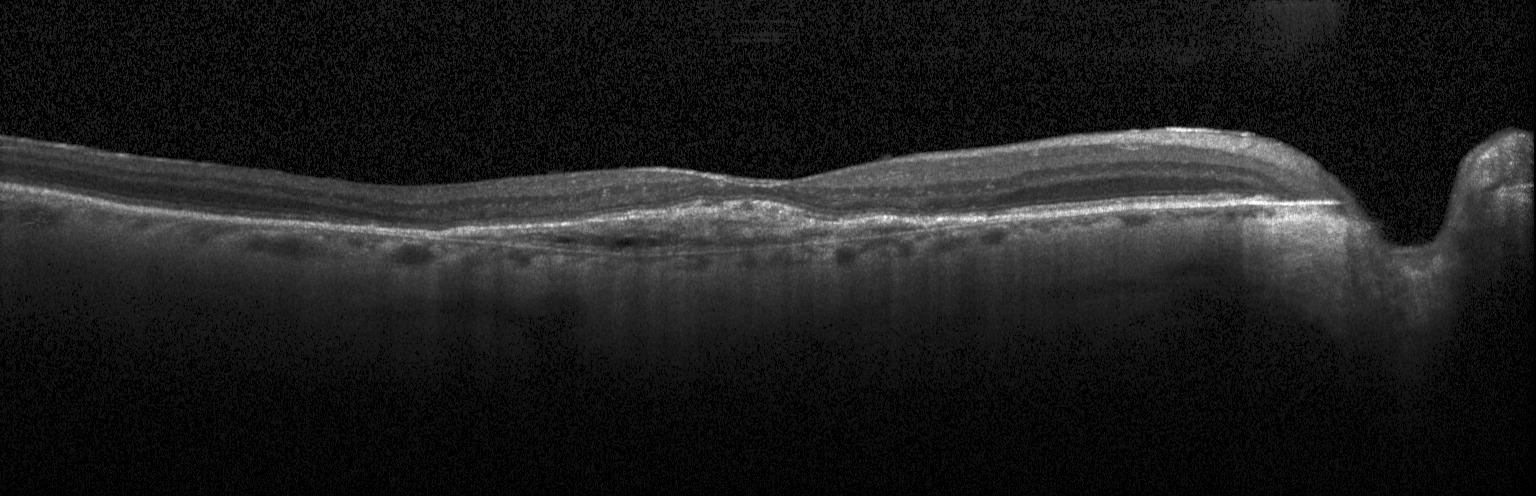
Instrument: Heidelberg Spectralis. OCT line scan. Diagnosis: choroidal neovascularization (CNV).